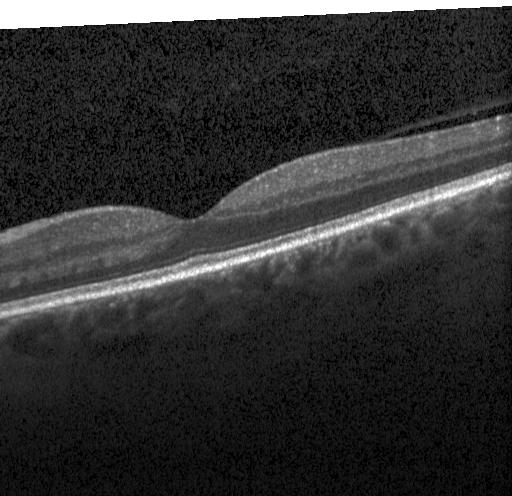

Impression: no CNV, DME, or drusen.